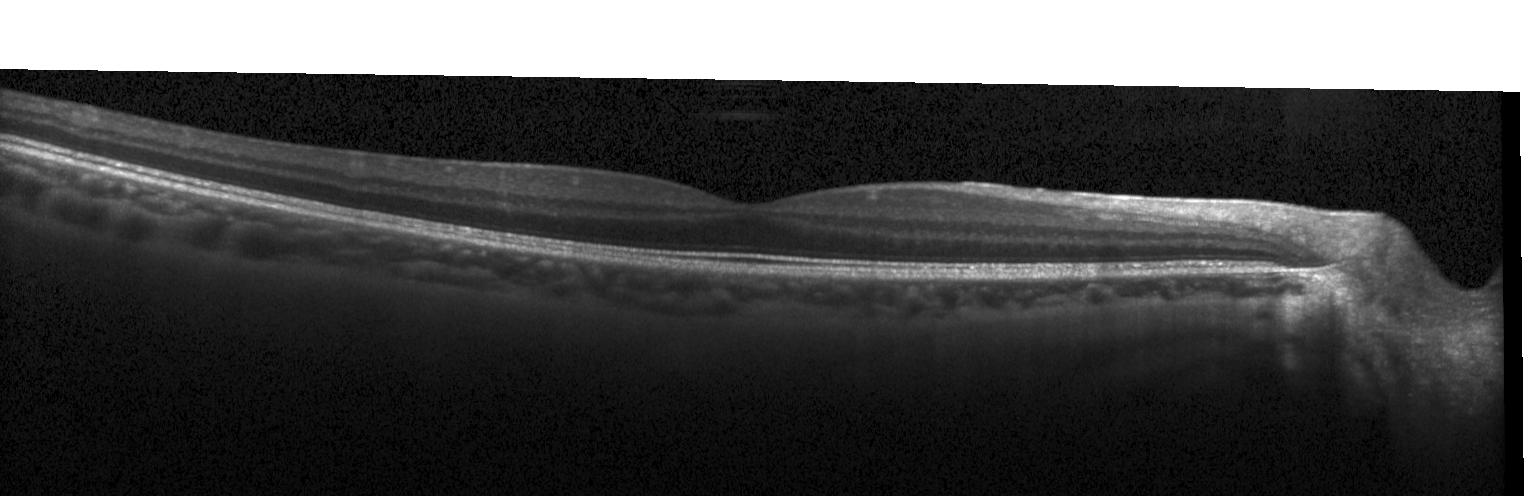
OCT finding: no evidence of choroidal neovascularization, diabetic macular edema, or drusen.